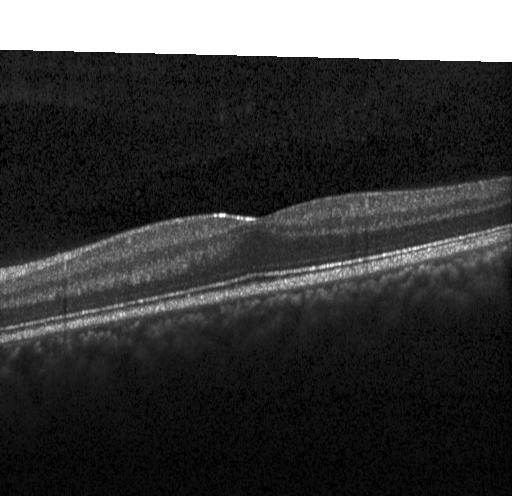
Acquired on a Heidelberg Spectralis. Optical coherence tomography B-scan — Finding: no choroidal neovascularization, no diabetic macular edema, and no drusen.